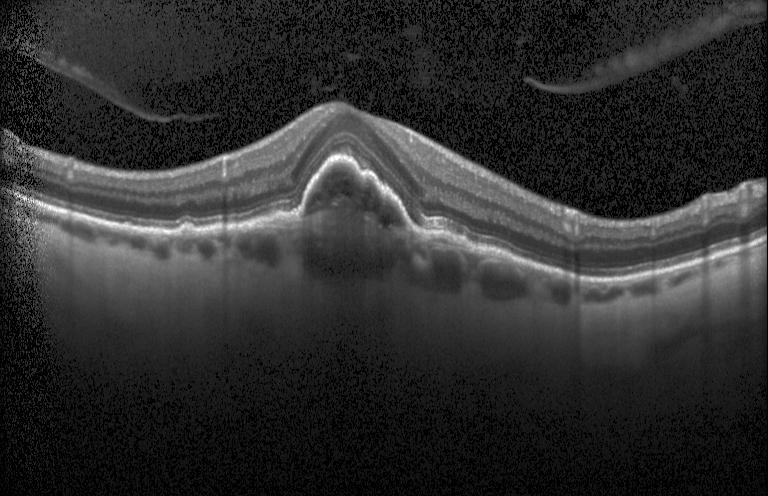
OCT B-scan
Diagnosis: choroidal neovascularization.